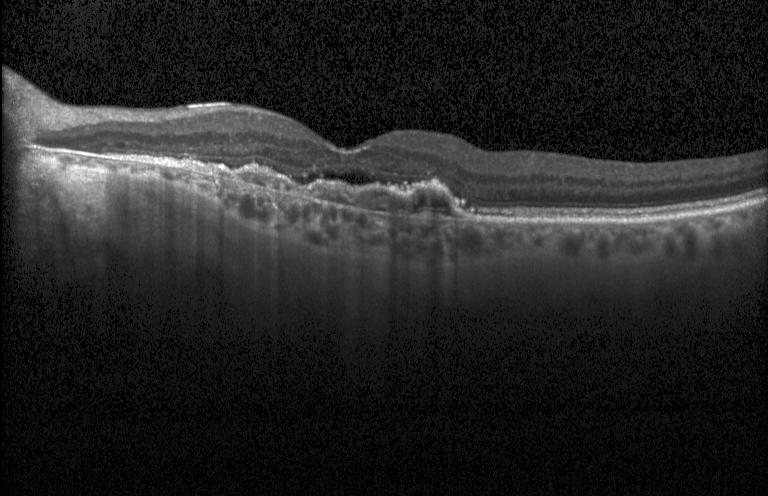 Optical coherence tomography scan, centered on the fovea, spectral-domain optical coherence tomography, Heidelberg Spectralis.
Impression: a choroidal neovascular membrane.